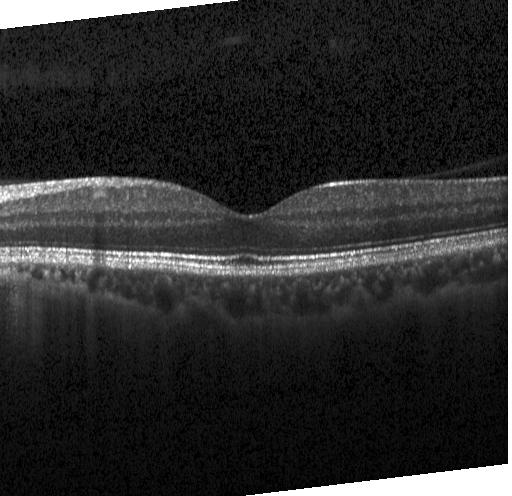

Acquired on a Heidelberg Spectralis; optical coherence tomography B-scan.
Impression: neither choroidal neovascularization, diabetic macular edema, nor drusen.